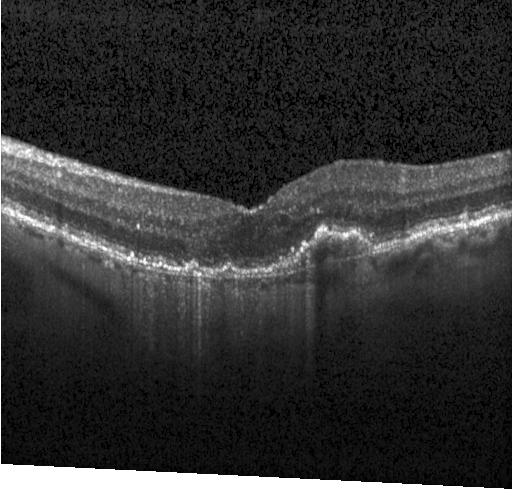 Retinal OCT cross-section. Heidelberg Spectralis OCT system. Centered on the fovea. Spectral-domain optical coherence tomography. The scan shows choroidal neovascularization (CNV).